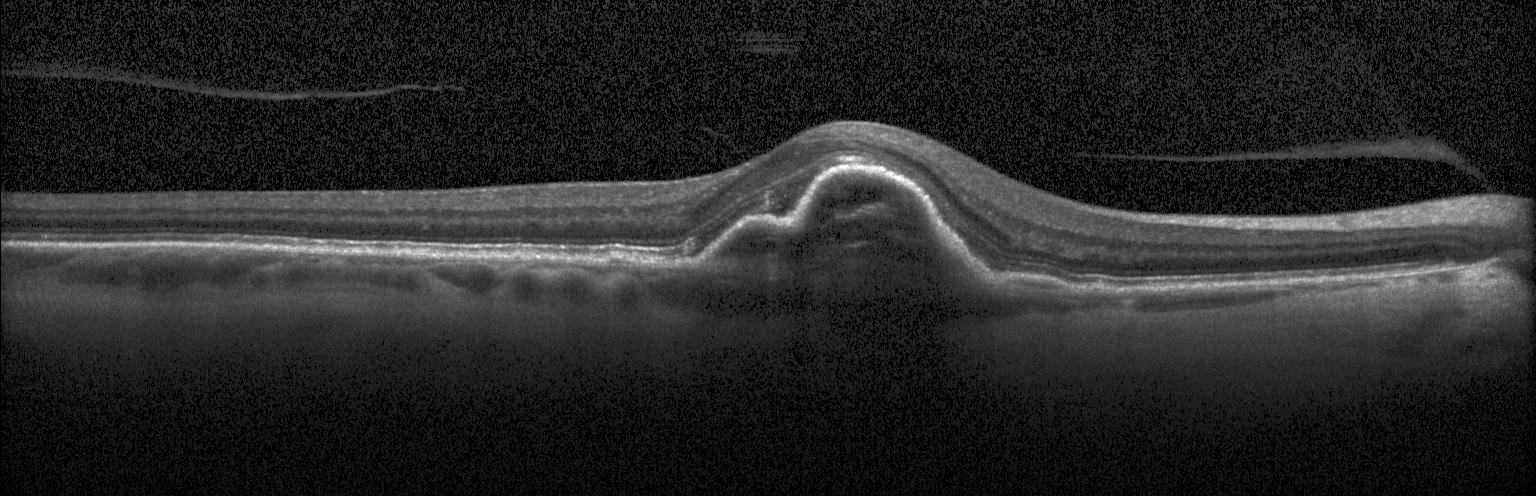
Impression: a choroidal neovascular membrane.